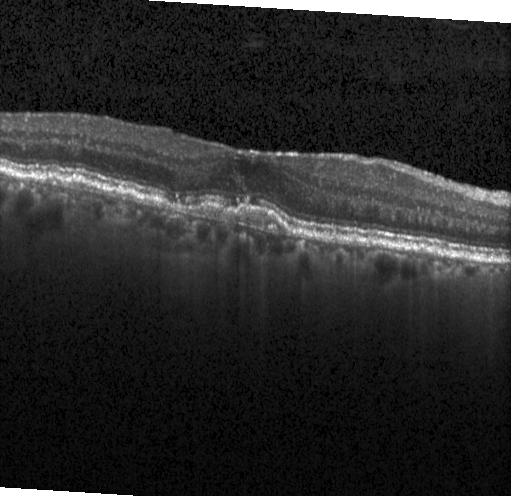

OCT B-scan; horizontal scan through the fovea. Diagnosis: a choroidal neovascular membrane.